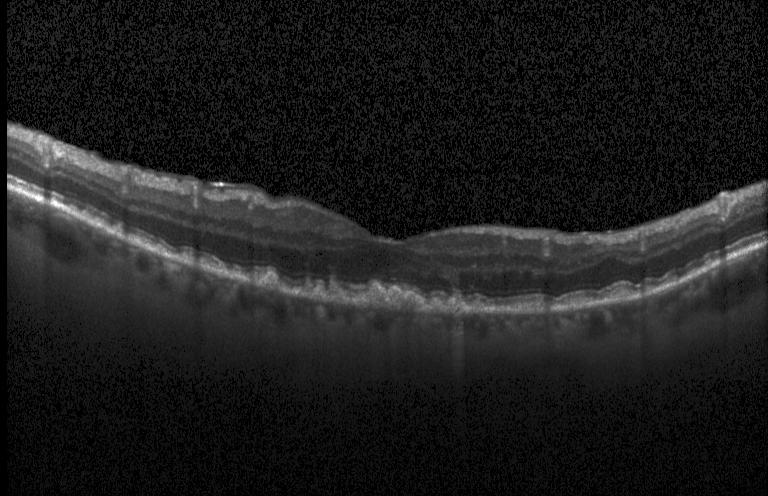 Retinal OCT cross-section
Impression: drusen.